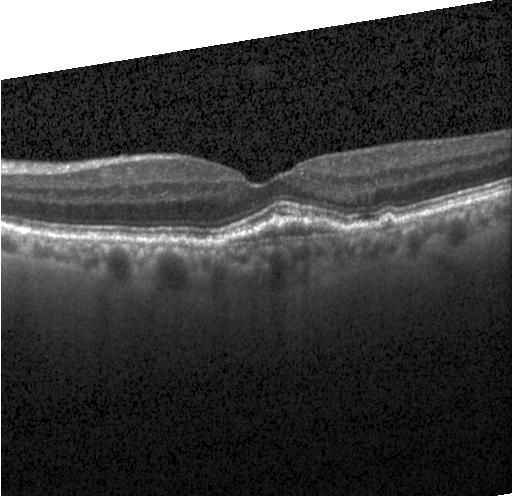 OCT line scan; instrument: Heidelberg Spectralis; macular scan; spectral-domain OCT. Macular OCT: a choroidal neovascular membrane.